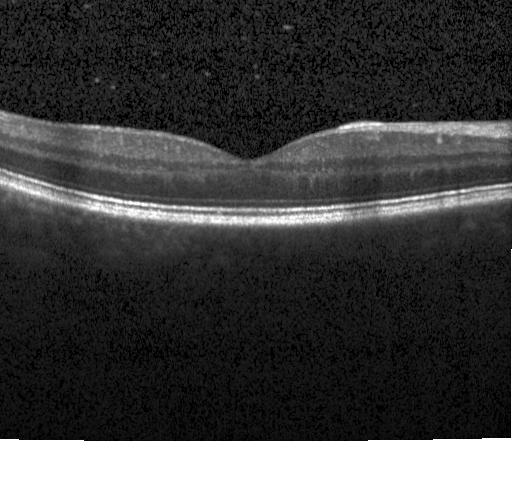
Optical coherence tomography scan; spectral-domain OCT; Heidelberg Spectralis
Diagnosis: neither choroidal neovascularization, diabetic macular edema, nor drusen.